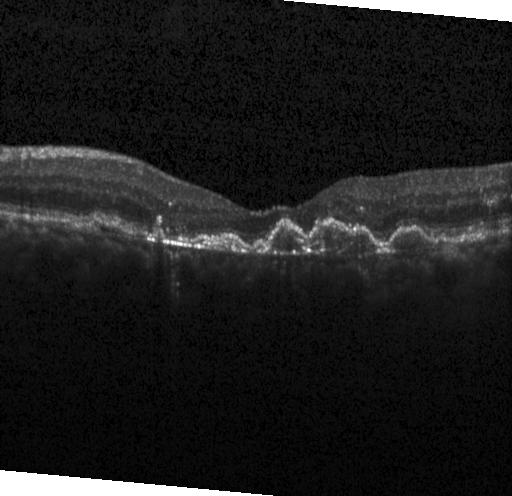 Retinal OCT cross-section. SD-OCT. OCT finding: a choroidal neovascular membrane.